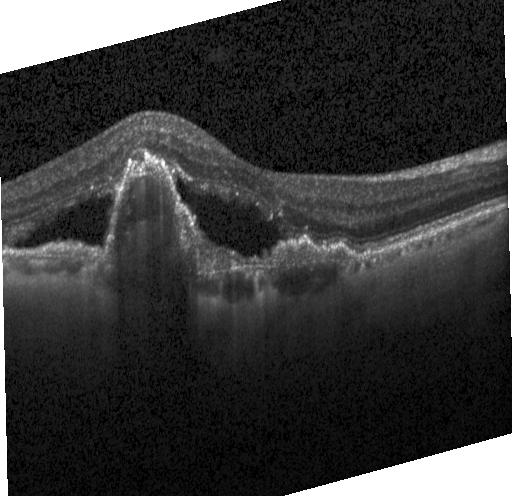
Macular OCT demonstrating choroidal neovascularization.